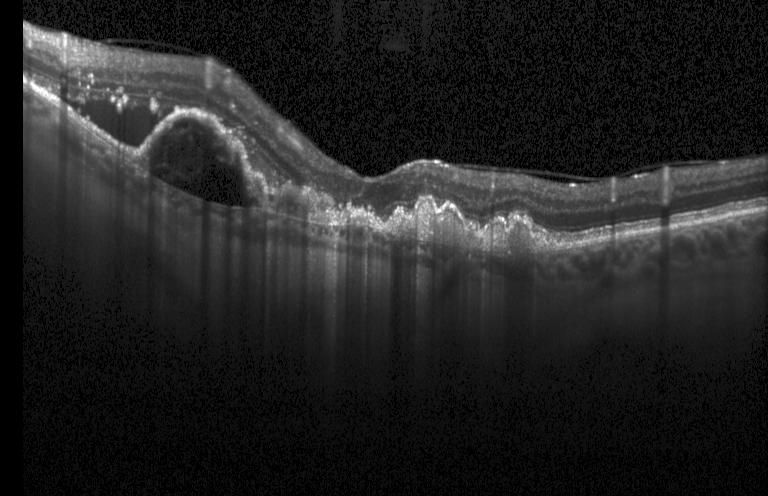 Dx: a choroidal neovascular membrane.